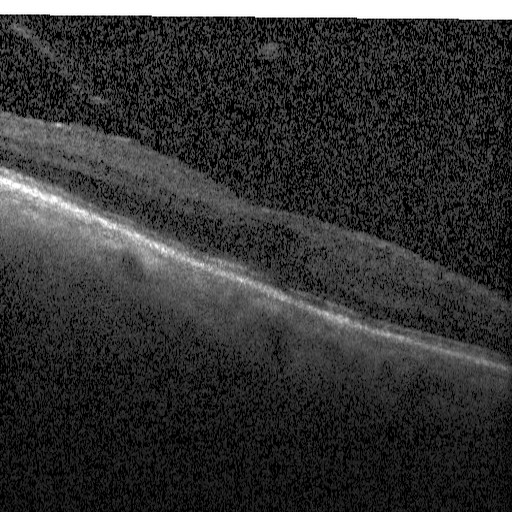
Optical coherence tomography scan. Diagnosis: diabetic macular edema.